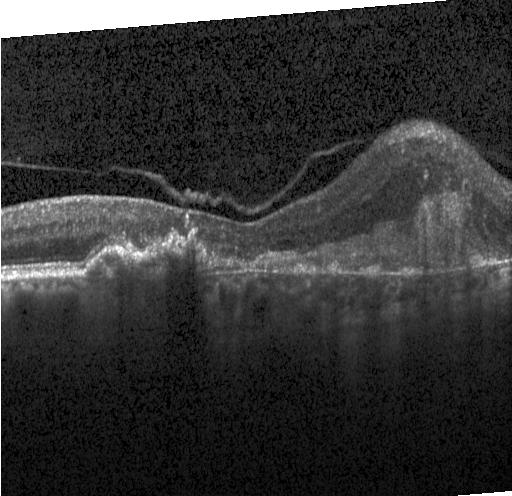

Macular OCT demonstrating CNV.